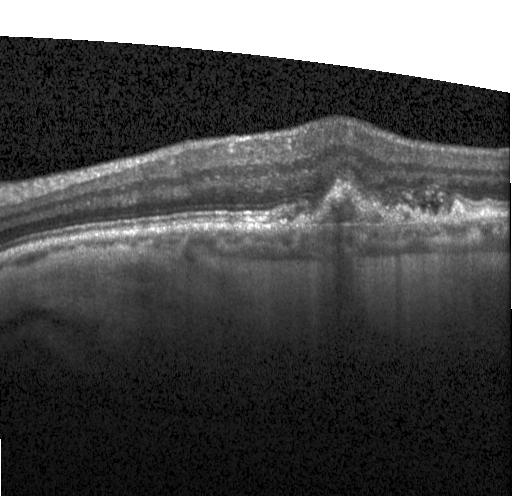

Heidelberg Spectralis OCT system. Spectral-domain optical coherence tomography. Retinal OCT cross-section.
OCT finding: choroidal neovascularization (CNV).